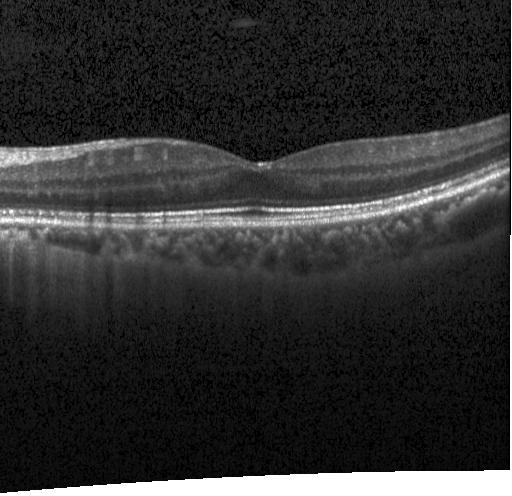
Impression: no choroidal neovascularization, diabetic macular edema, or drusen.